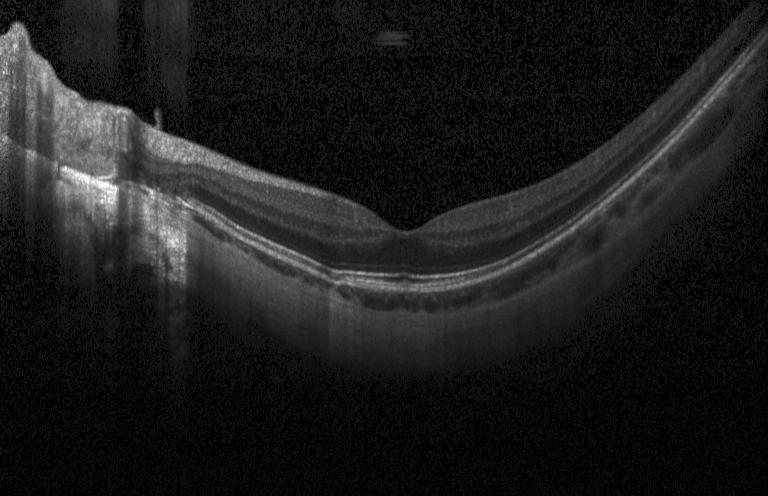

Diagnosis: neither CNV, DME, nor drusen.